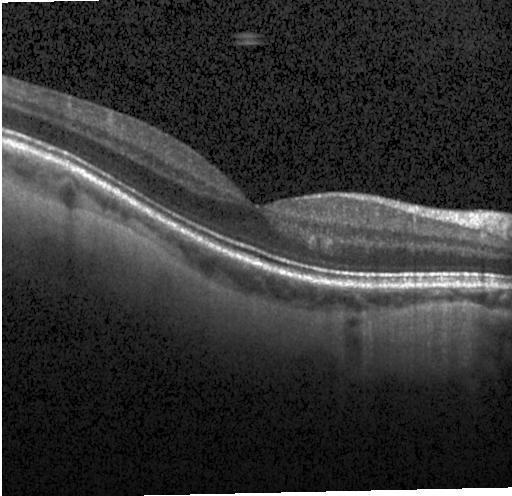 Optical coherence tomography scan · instrument: Heidelberg Spectralis · horizontal scan through the fovea
Assessment: no CNV, DME, or drusen.